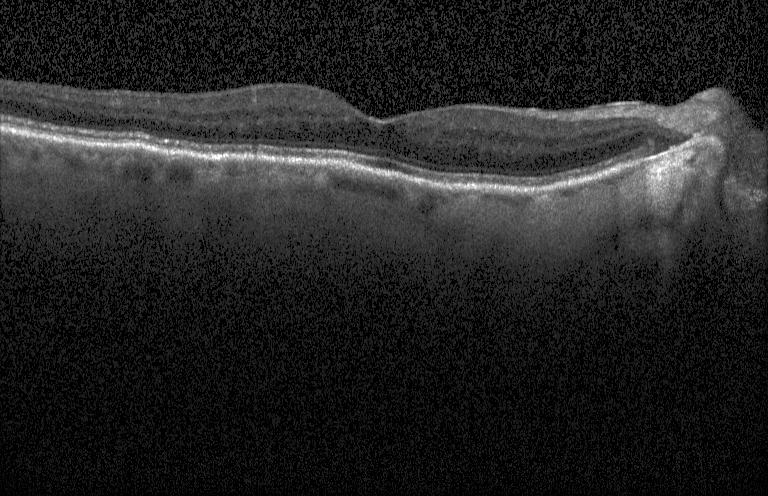

Spectral-domain OCT; instrument: Heidelberg Spectralis; horizontal scan through the fovea; OCT line scan.
No choroidal neovascularization, diabetic macular edema, or drusen.